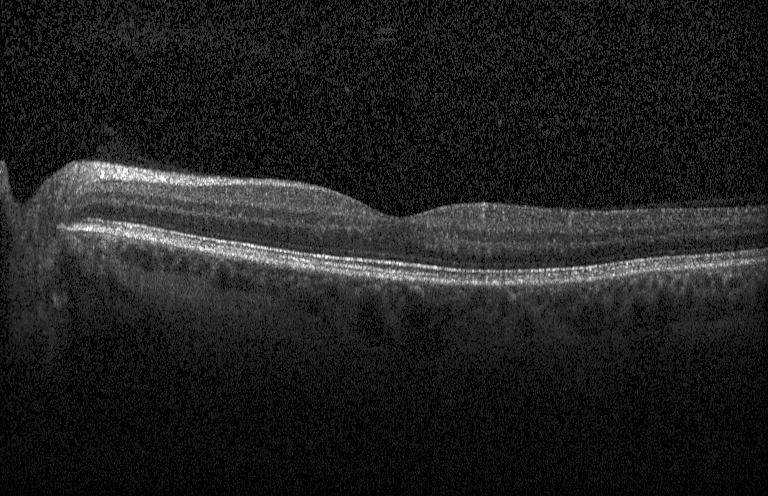
Spectral-domain OCT B-scan: neither CNV, DME, nor drusen.